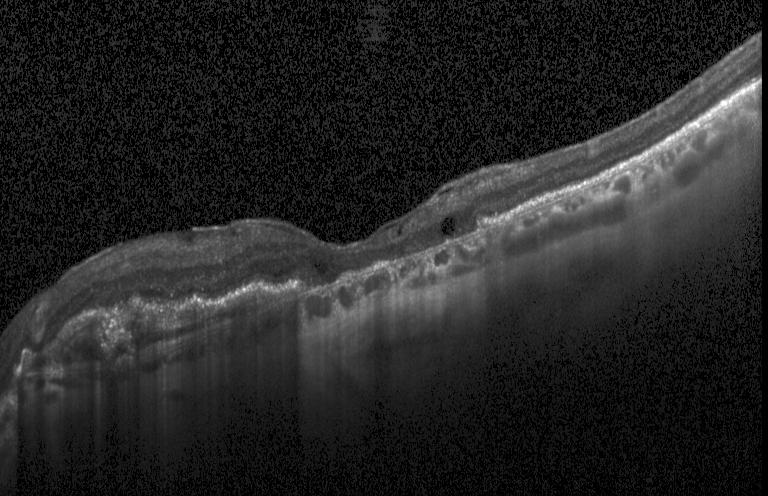 Instrument: Heidelberg Spectralis. Optical coherence tomography B-scan. This B-scan demonstrates a choroidal neovascular membrane.